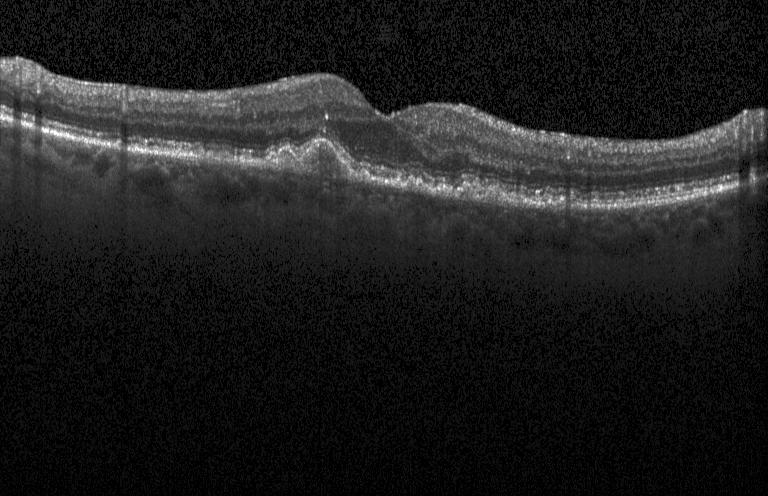

Acquired on a Heidelberg Spectralis, through the macula, optical coherence tomography B-scan — Diagnosis: multiple drusen.